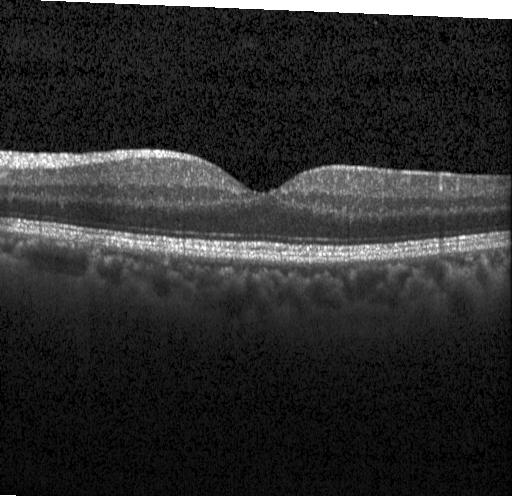

Instrument: Heidelberg Spectralis. Centered on the fovea. Optical coherence tomography B-scan. Spectral-domain optical coherence tomography
Impression: neither CNV, DME, nor drusen.